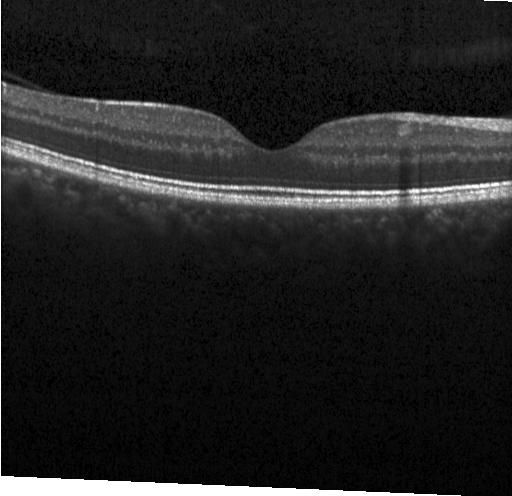
OCT B-scan — Impression: no evidence of choroidal neovascularization, diabetic macular edema, or drusen.